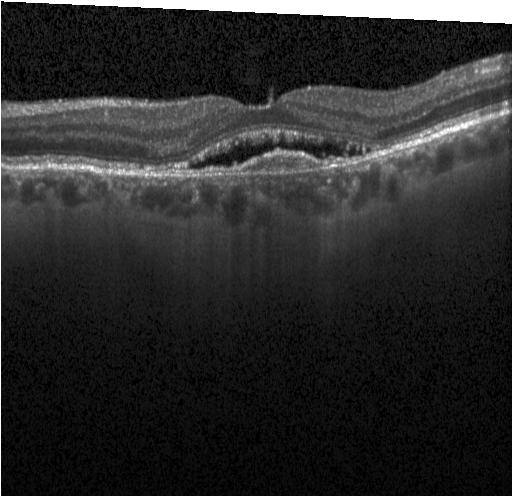

The scan shows choroidal neovascularization (CNV).